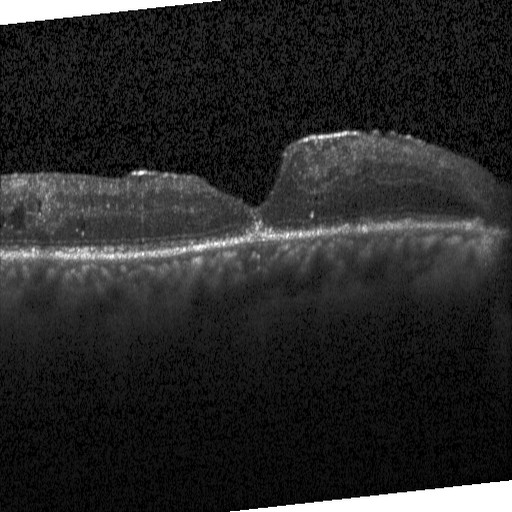
OCT B-scan; horizontal scan through the fovea; spectral-domain optical coherence tomography — Diabetic macular edema (DME).